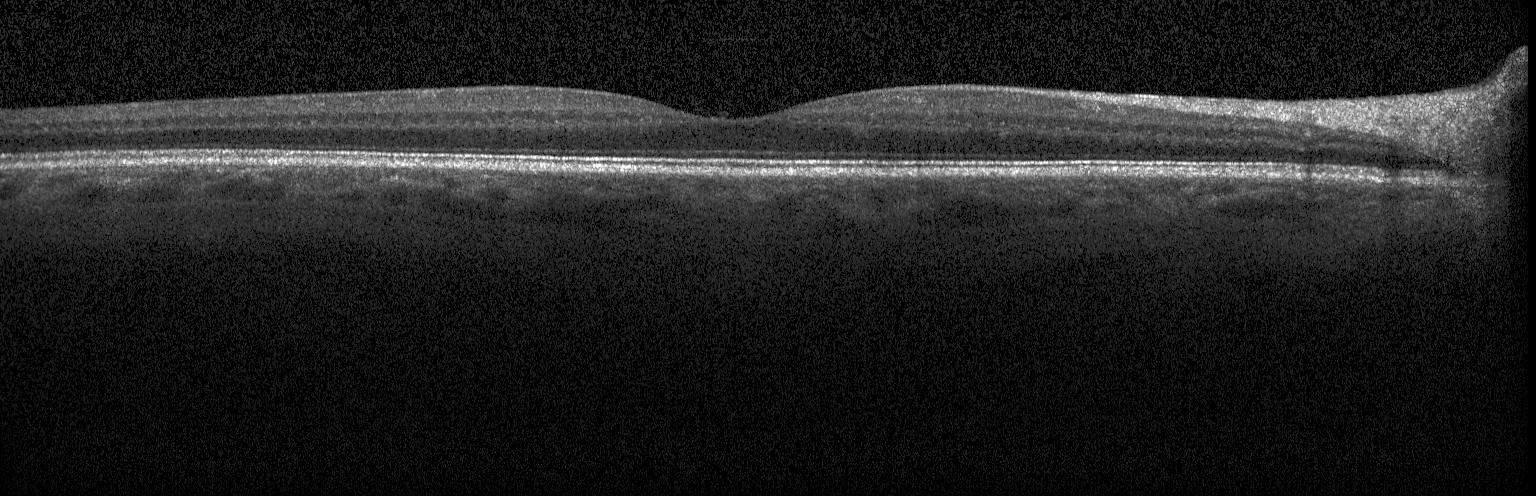
Optical coherence tomography scan — No choroidal neovascularization, no diabetic macular edema, and no drusen.